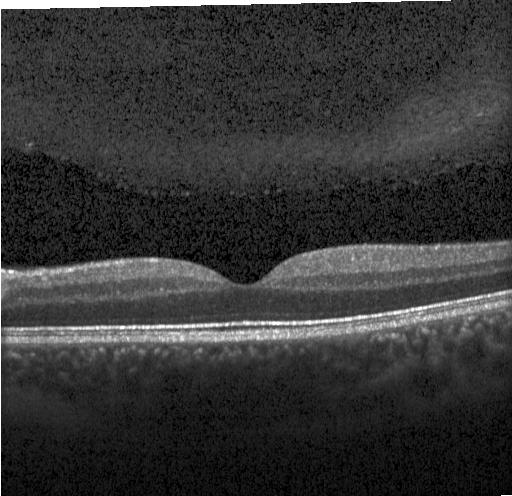
Retinal OCT cross-section. Spectral-domain optical coherence tomography. Macular scan. Acquired on a Heidelberg Spectralis — Diagnosis: no choroidal neovascularization, diabetic macular edema, or drusen.